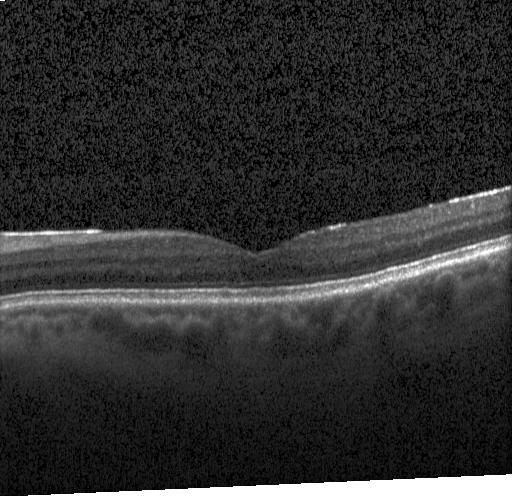
Macular OCT demonstrating no choroidal neovascularization, no diabetic macular edema, and no drusen.